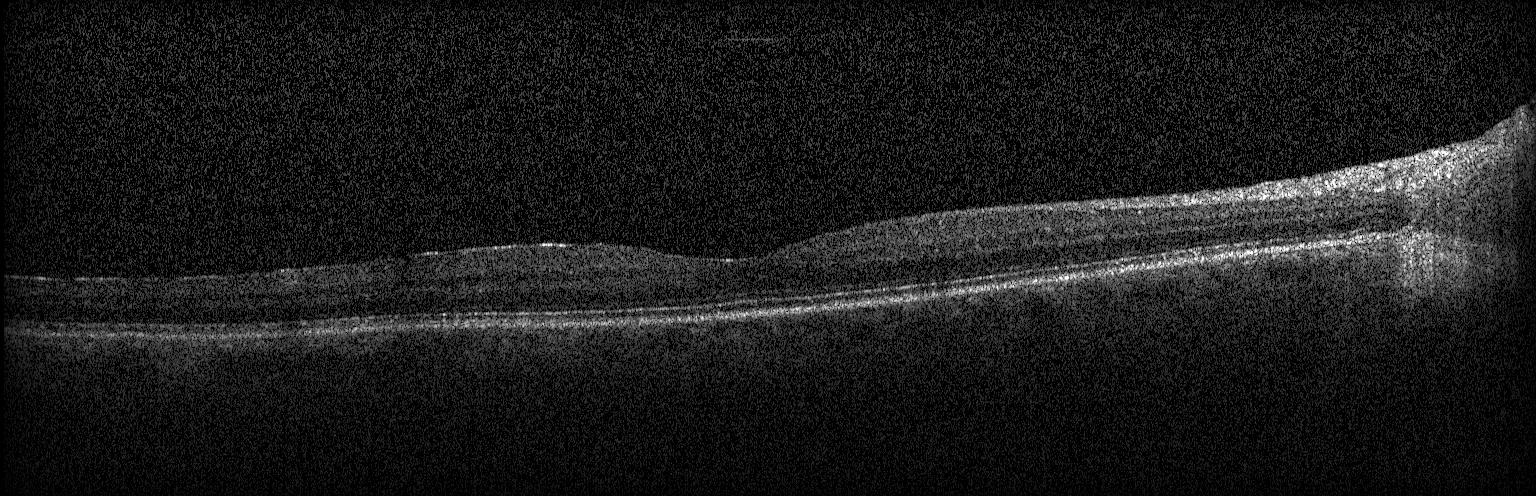

Fovea-centered, acquired on a Heidelberg Spectralis, SD-OCT, OCT line scan. Finding: neither choroidal neovascularization, diabetic macular edema, nor drusen.